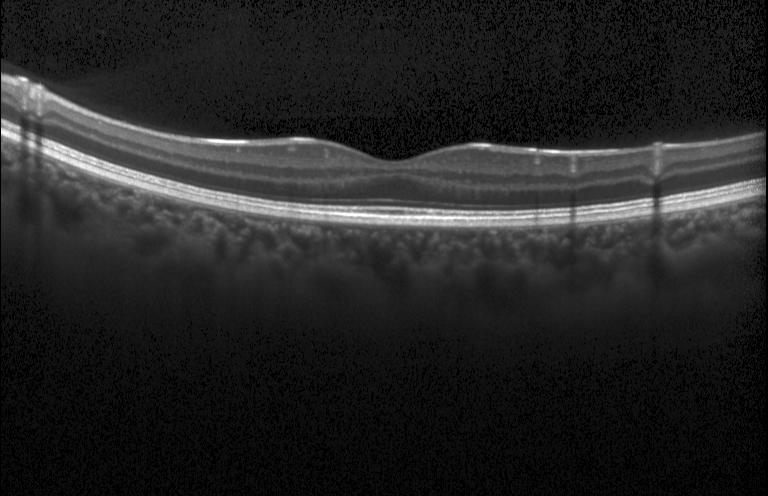

SD-OCT. Acquired on a Heidelberg Spectralis. Optical coherence tomography scan. Centered on the fovea. The scan shows no choroidal neovascularization, diabetic macular edema, or drusen.